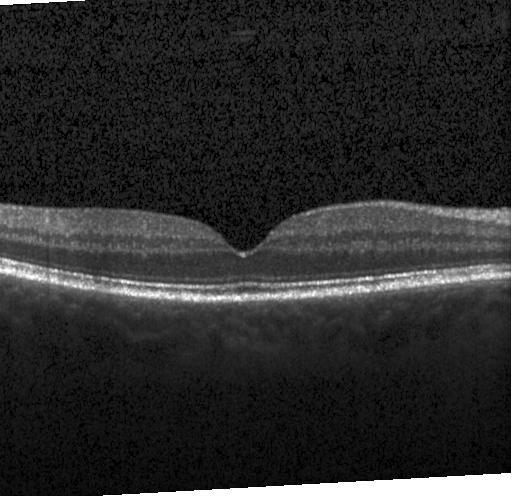 Heidelberg Spectralis, spectral-domain optical coherence tomography, macular scan, OCT line scan
Impression: no choroidal neovascularization, diabetic macular edema, or drusen.